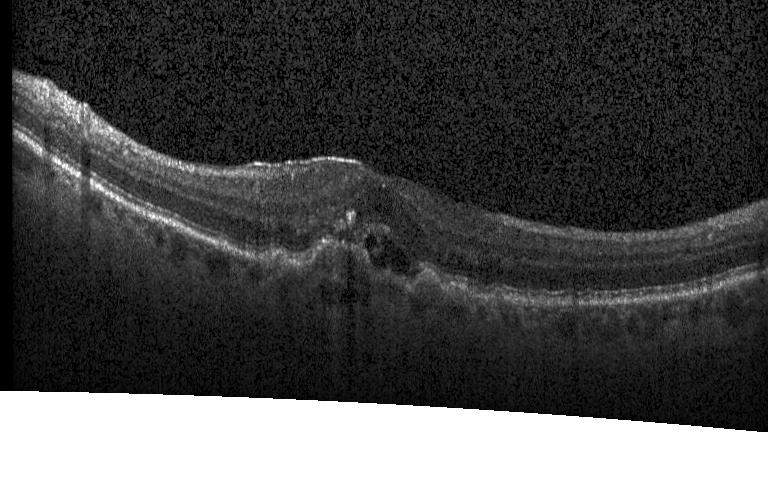 This B-scan demonstrates a choroidal neovascular membrane.